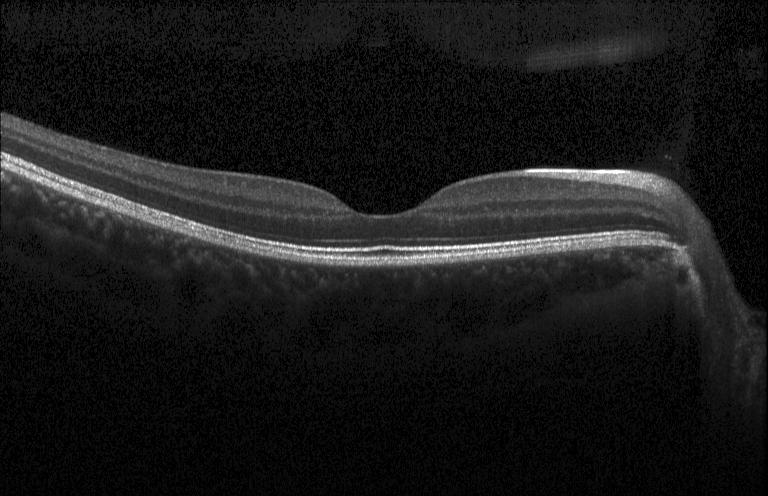
The scan shows no CNV, no DME, and no drusen.